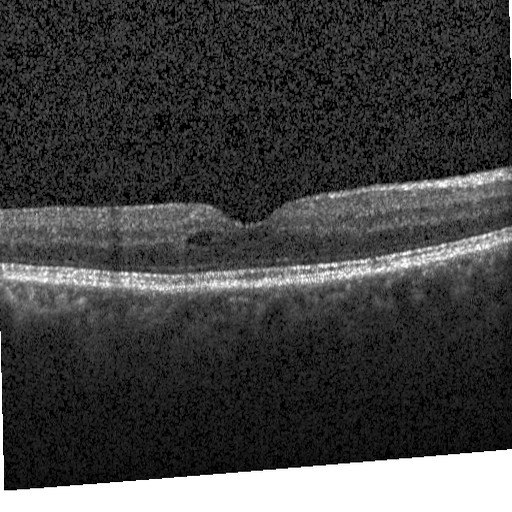
Optical coherence tomography B-scan.
Finding: diabetic macular edema.